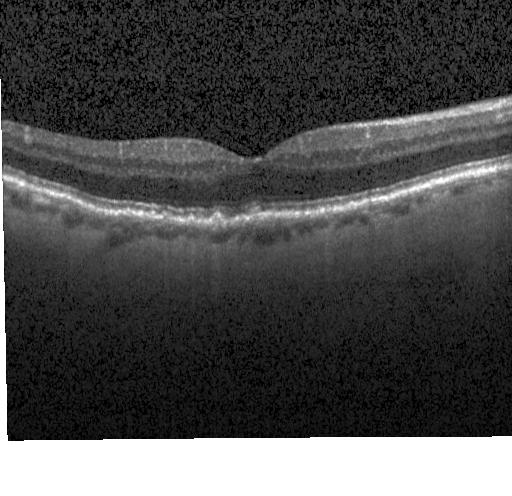

Retinal OCT cross-section — Impression: multiple drusen.